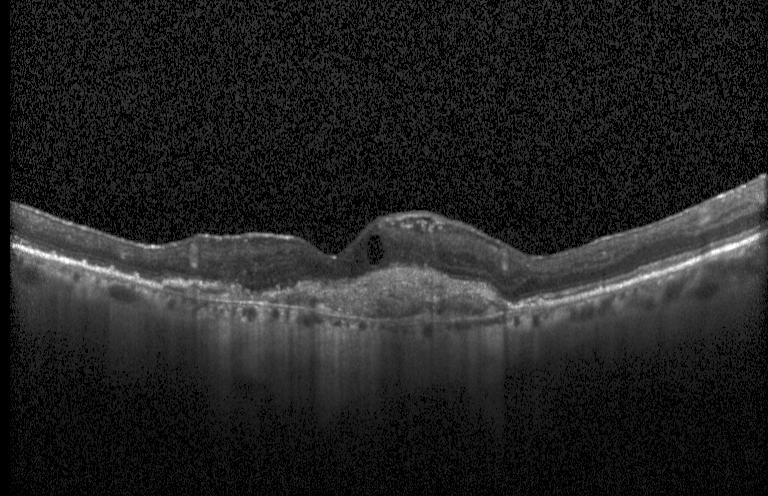

Spectral-domain OCT · through the macula · OCT line scan
OCT finding: choroidal neovascularization (CNV).